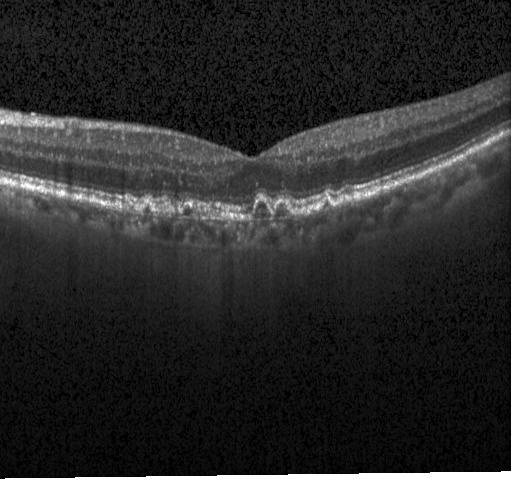 Optical coherence tomography B-scan · Heidelberg Spectralis OCT system · horizontal scan through the fovea · spectral-domain optical coherence tomography — Finding: sub-RPE drusenoid deposits.